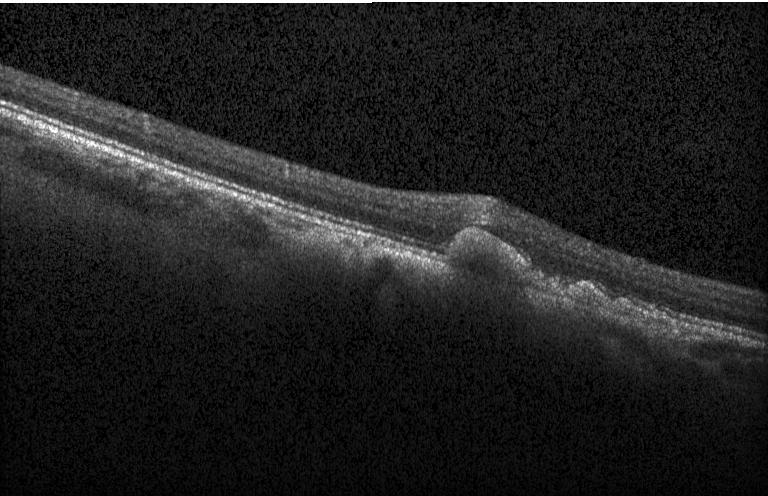

Optical coherence tomography B-scan — A choroidal neovascular membrane.